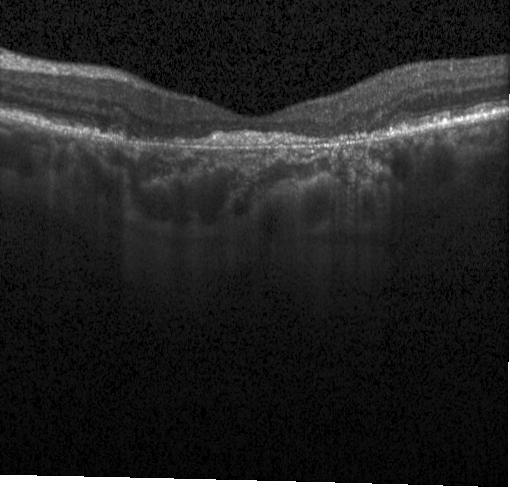 Spectral-domain optical coherence tomography; optical coherence tomography B-scan; Heidelberg Spectralis; horizontal scan through the fovea — OCT finding: a choroidal neovascular membrane.